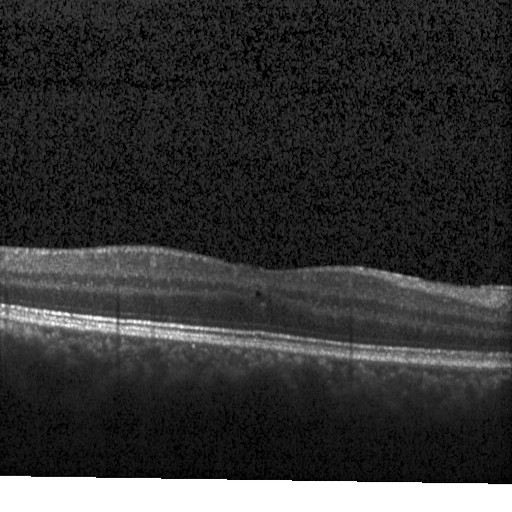

OCT finding: diabetic macular edema.